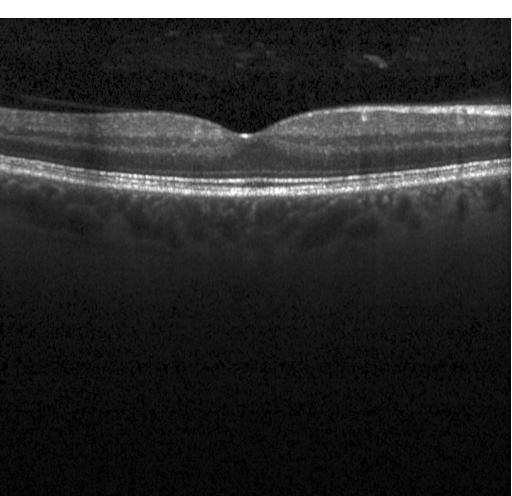
Retinal OCT cross-section
Impression: no choroidal neovascularization, diabetic macular edema, or drusen.